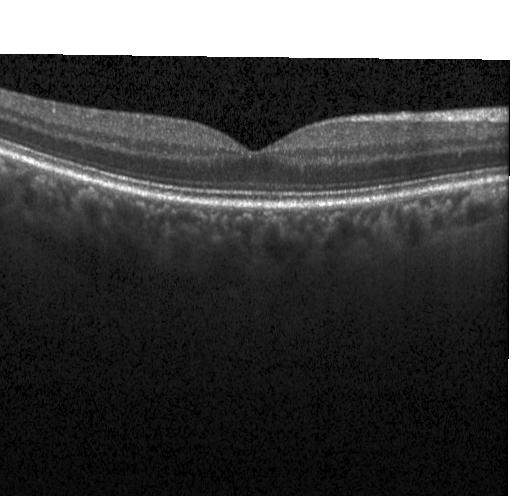

OCT finding: no CNV, DME, or drusen.